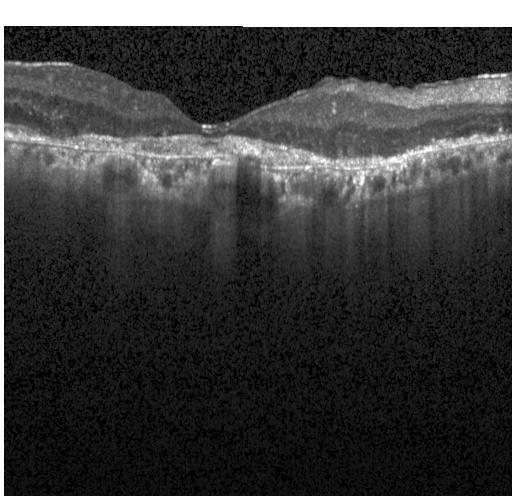
Retinal OCT B-scan, fovea-centered, spectral-domain optical coherence tomography. Diagnosis: choroidal neovascularization (CNV).